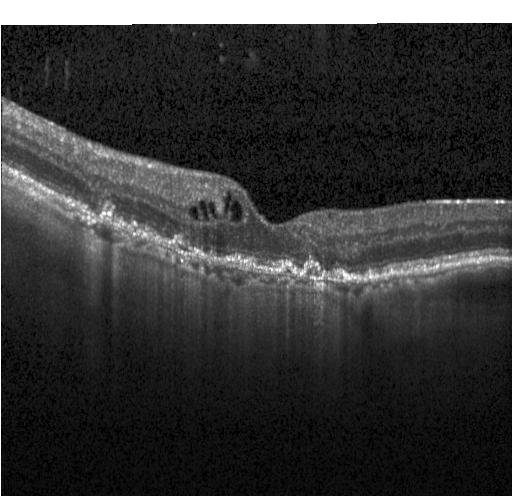
Finding: a choroidal neovascular membrane.